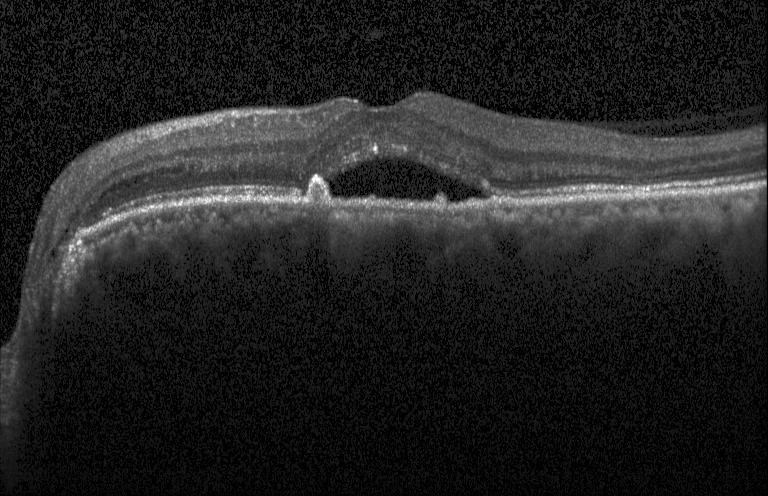
Macular scan; acquired on a Heidelberg Spectralis; SD-OCT; optical coherence tomography B-scan.
Impression: choroidal neovascularization (CNV).